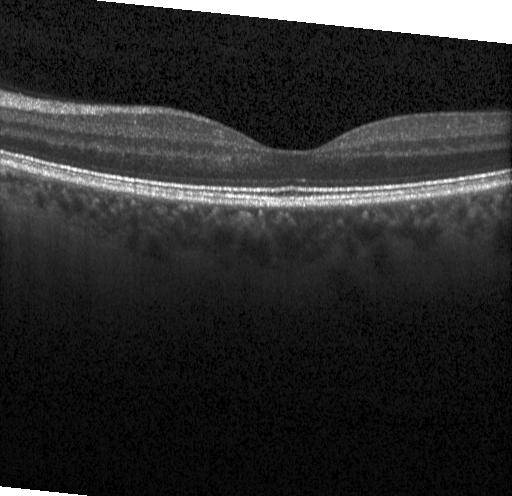
SD-OCT; optical coherence tomography scan; instrument: Heidelberg Spectralis.
No CNV, no DME, and no drusen.